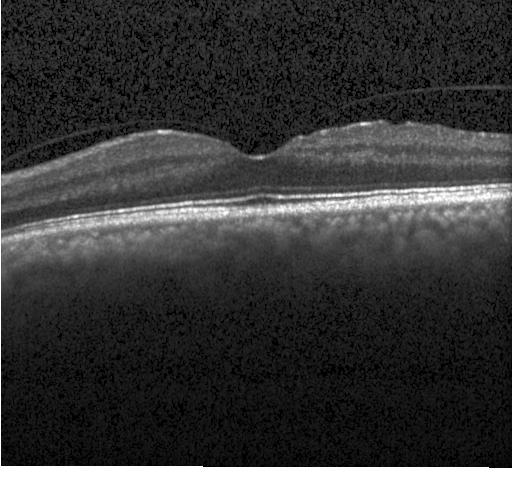

Centered on the fovea; optical coherence tomography B-scan.
Finding: no evidence of choroidal neovascularization, diabetic macular edema, or drusen.